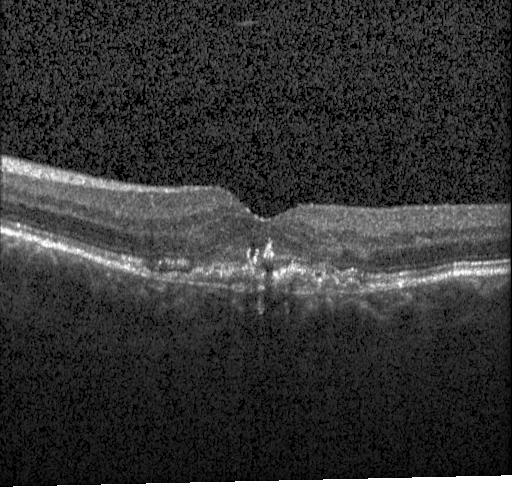

Macular scan, OCT B-scan, Heidelberg Spectralis OCT system, spectral-domain OCT.
Impression: CNV.